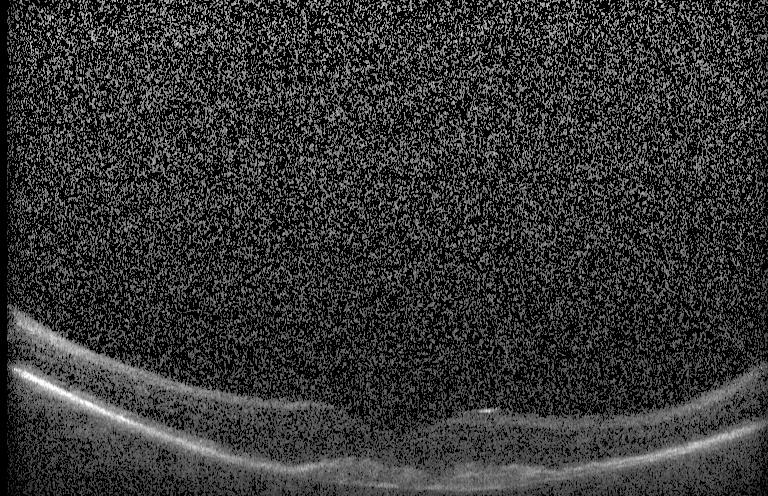
This B-scan demonstrates a choroidal neovascular membrane.